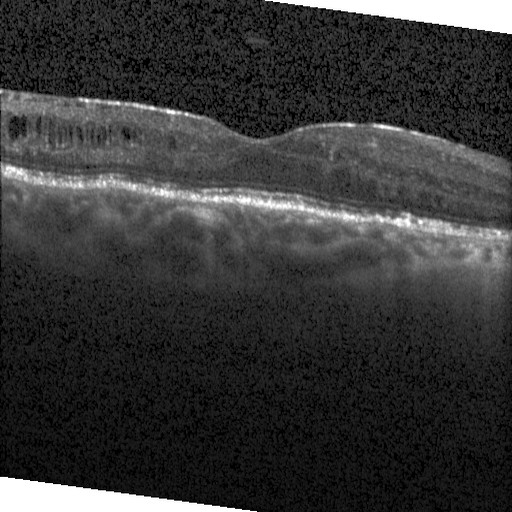
Macular OCT demonstrating DME.